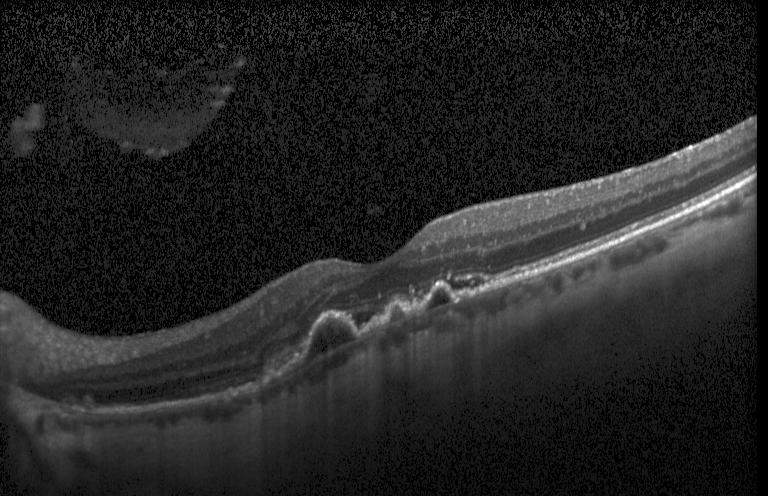

Macular OCT demonstrating a choroidal neovascular membrane.